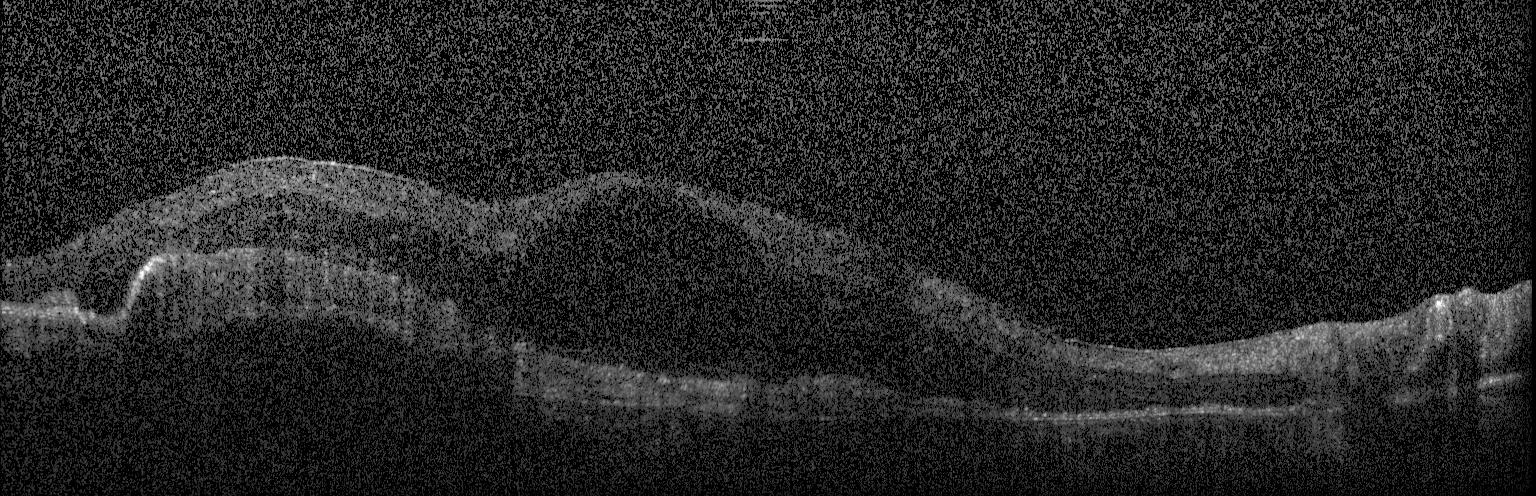
Macular OCT: choroidal neovascularization (CNV).